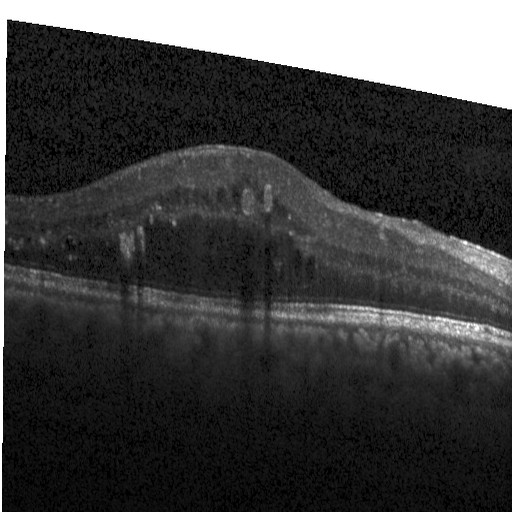 Instrument: Heidelberg Spectralis, spectral-domain OCT, retinal OCT cross-section, centered on the fovea. Diagnosis: diabetic macular edema.